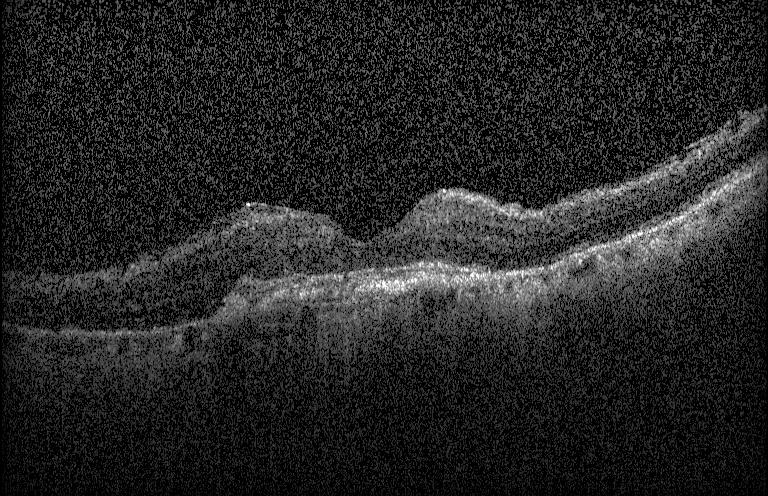 Spectral-domain optical coherence tomography. OCT B-scan. Instrument: Heidelberg Spectralis.
The scan shows a choroidal neovascular membrane.